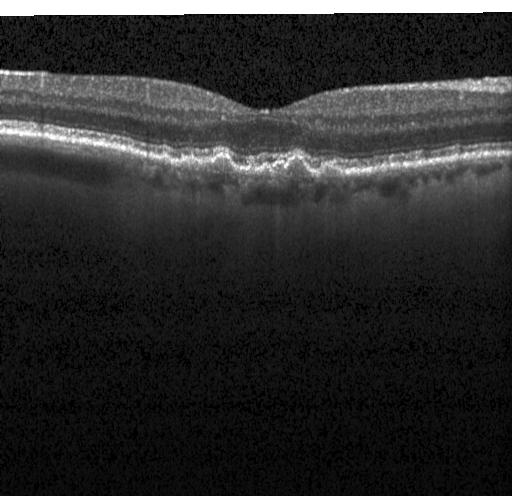 OCT B-scan showing drusen.